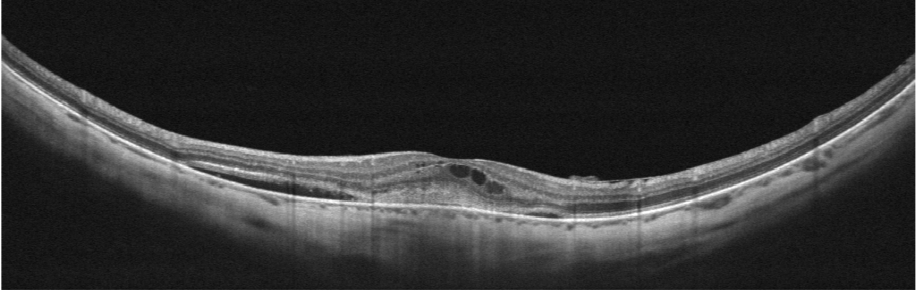 Assessment: AMD.